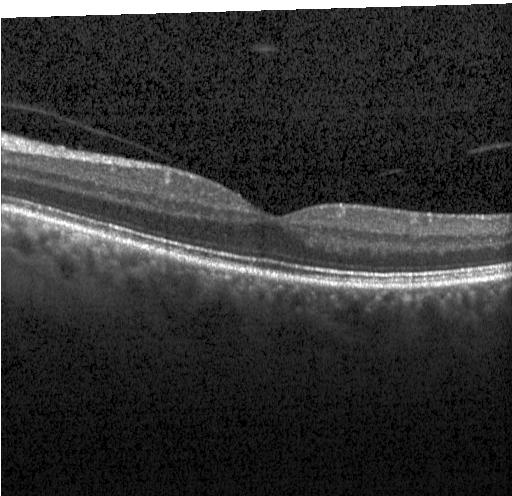

Optical coherence tomography scan, spectral-domain optical coherence tomography
Impression: no choroidal neovascularization, diabetic macular edema, or drusen.